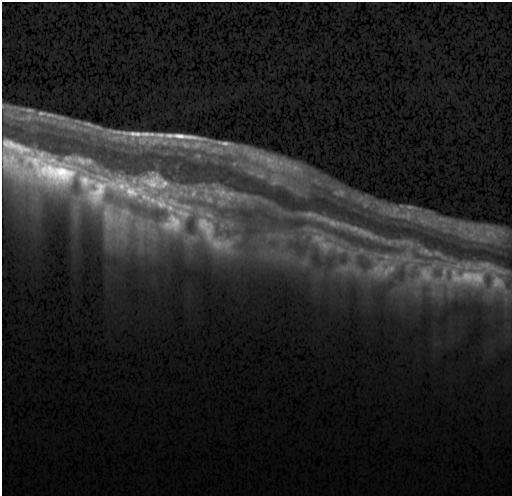

Acquired on a Heidelberg Spectralis, centered on the fovea, spectral-domain OCT, OCT line scan. The scan shows choroidal neovascularization.